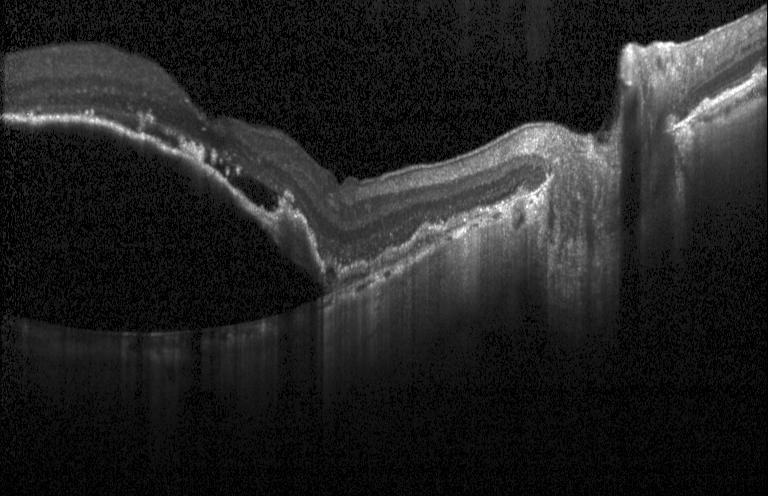

Retinal OCT B-scan — Assessment: CNV.